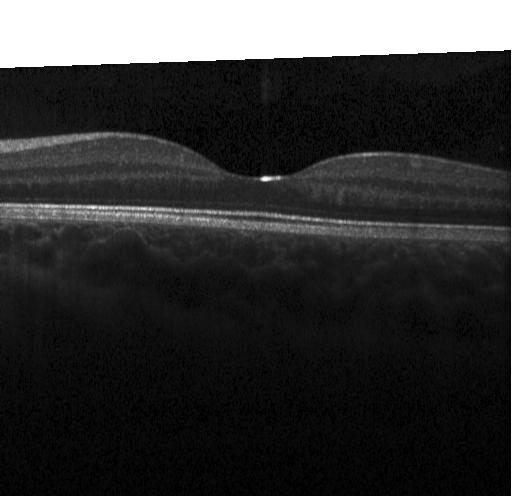

OCT line scan; Heidelberg Spectralis OCT system; spectral-domain optical coherence tomography; centered on the fovea — Impression: no choroidal neovascularization, no diabetic macular edema, and no drusen.